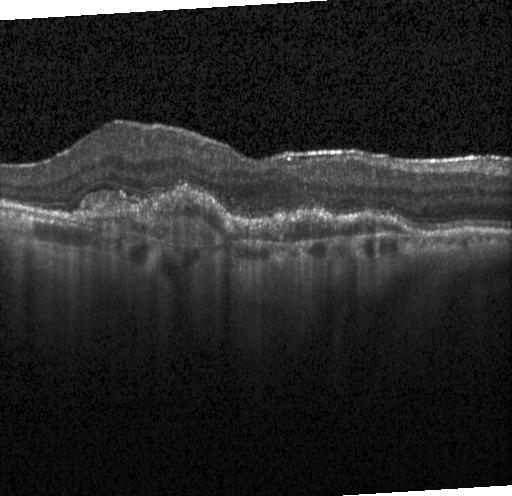
Optical coherence tomography B-scan — Diagnosis: a choroidal neovascular membrane.